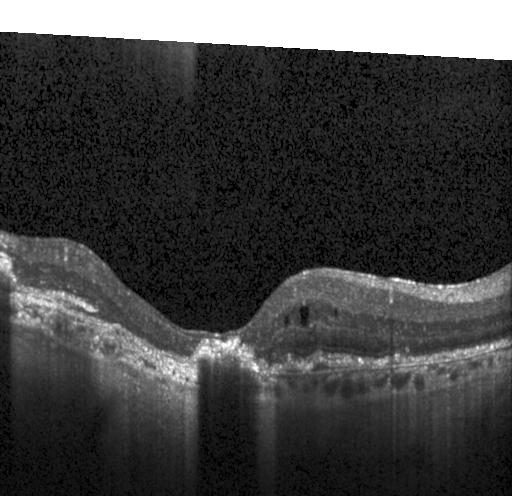 Optical coherence tomography scan. Dx: choroidal neovascularization (CNV).